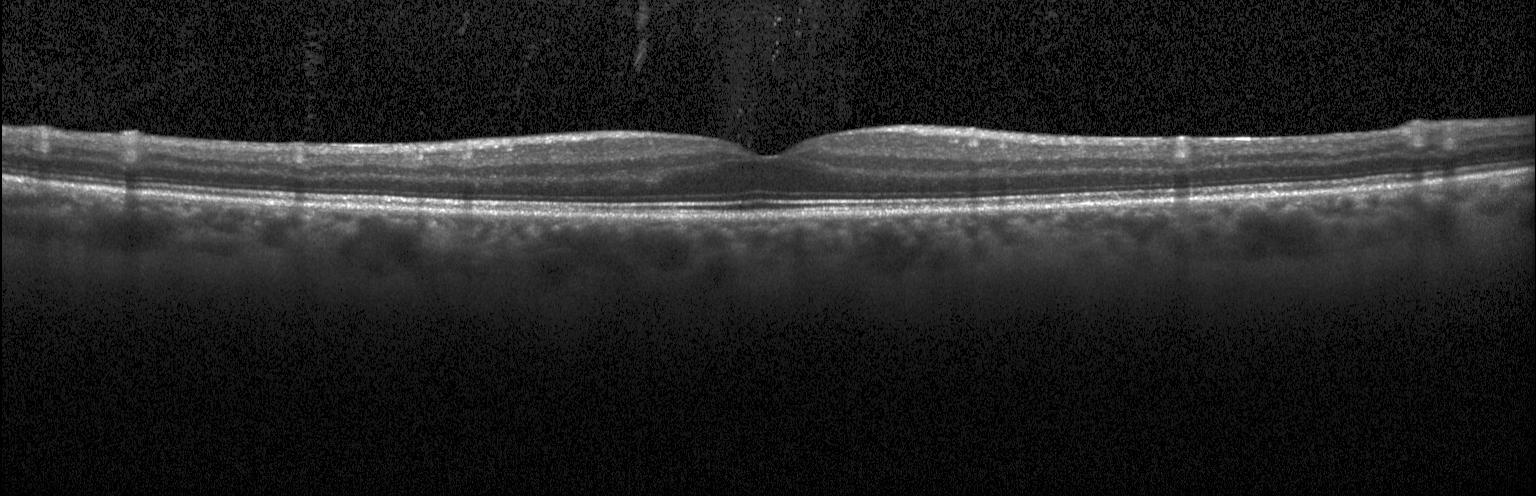
Retinal OCT cross-section; Heidelberg Spectralis; spectral-domain OCT. This B-scan demonstrates neither choroidal neovascularization, diabetic macular edema, nor drusen.